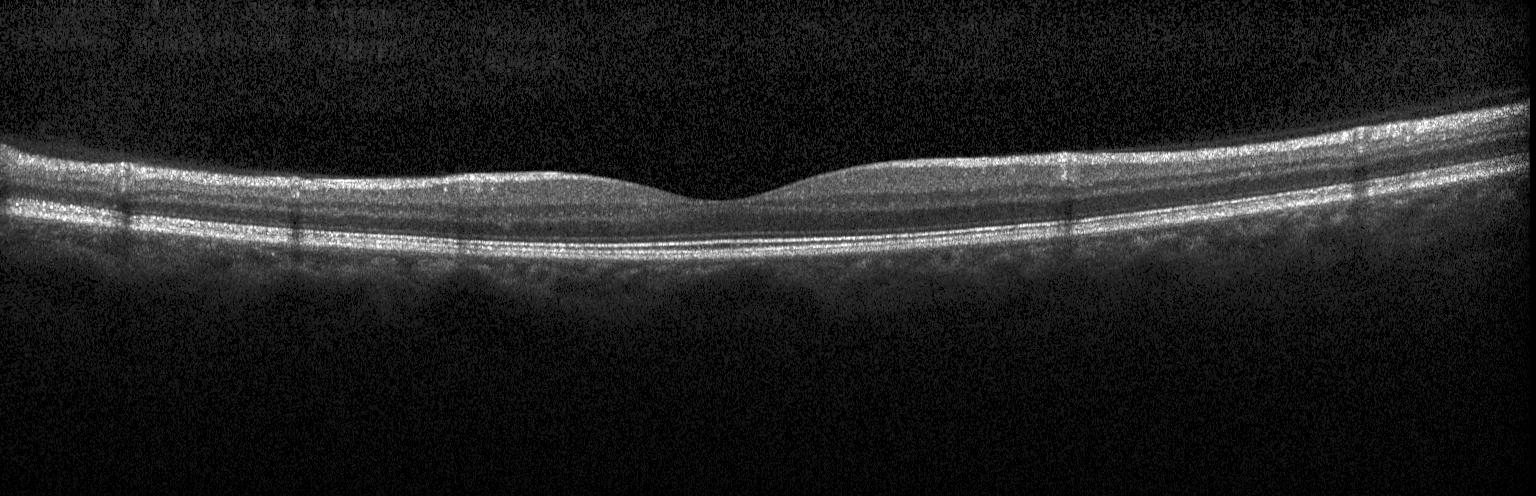
Spectral-domain OCT B-scan: no choroidal neovascularization, diabetic macular edema, or drusen.